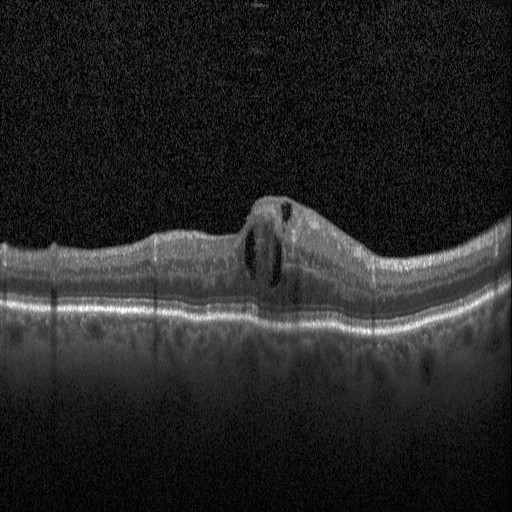

Optical coherence tomography B-scan; macular scan — Finding: diabetic macular edema (DME).